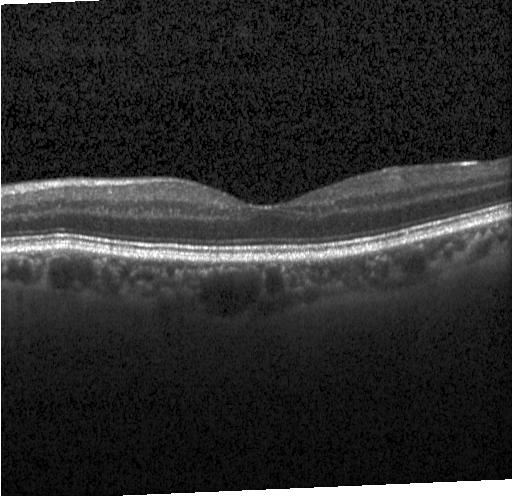

Neither choroidal neovascularization, diabetic macular edema, nor drusen.